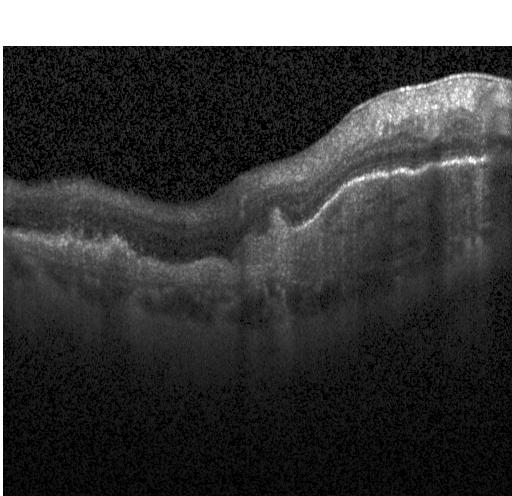
Heidelberg Spectralis · centered on the fovea · OCT line scan.
This B-scan demonstrates choroidal neovascularization.